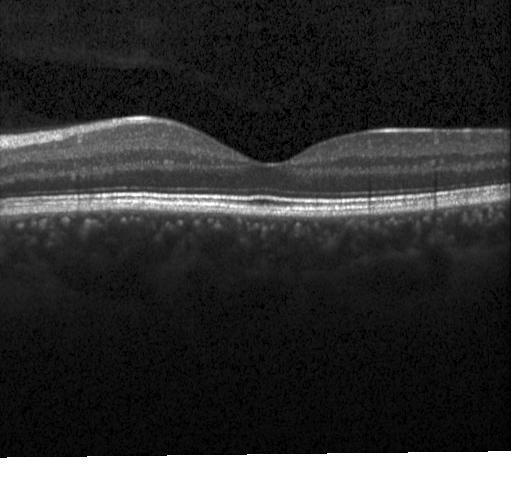
Spectral-domain OCT B-scan: no evidence of CNV, DME, or drusen.